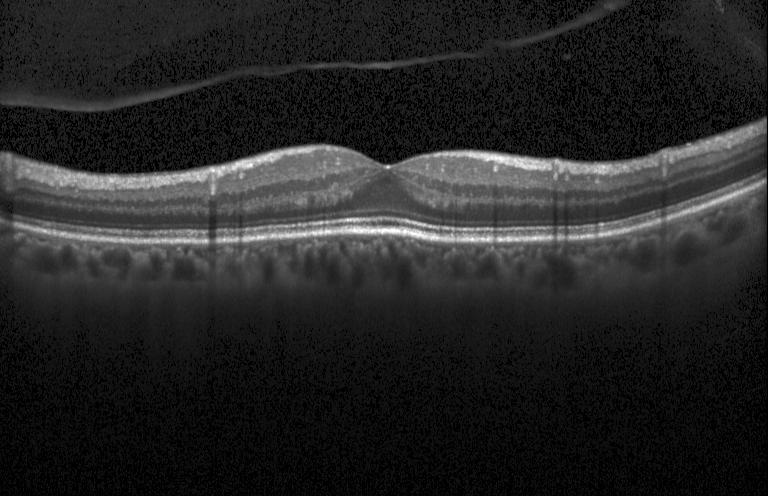 Heidelberg Spectralis OCT system. Spectral-domain OCT. Retinal OCT B-scan. Horizontal scan through the fovea.
Impression: no choroidal neovascularization, diabetic macular edema, or drusen.